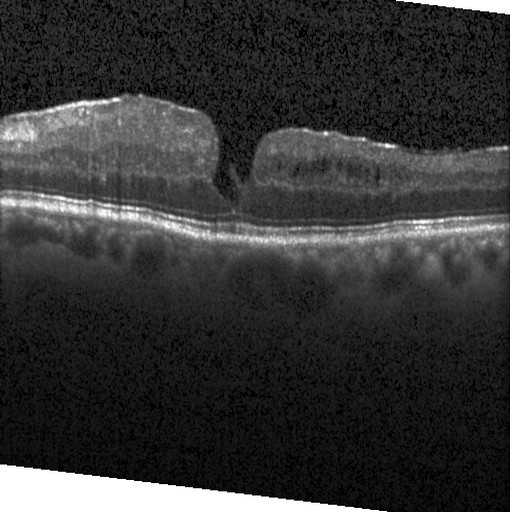
This B-scan demonstrates DME.